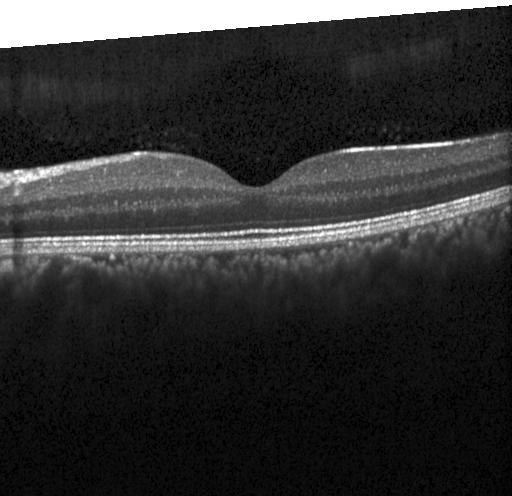
Diagnosis: no CNV, DME, or drusen.